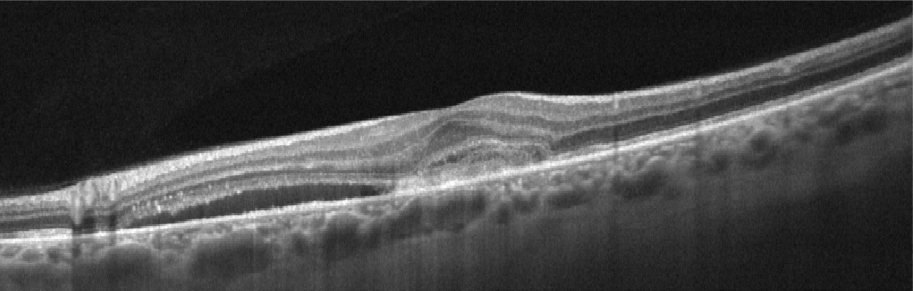 OCT B-scan — Age-related macular degeneration.